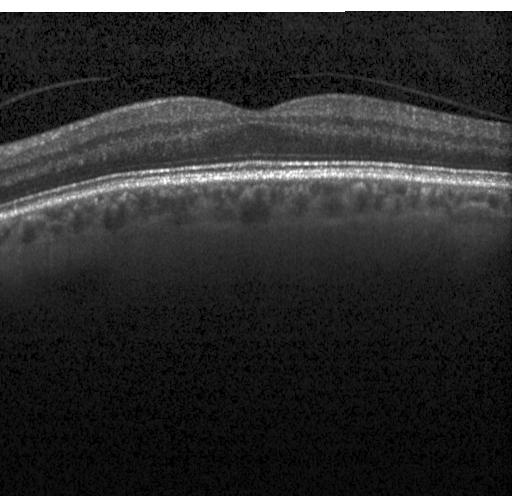

OCT line scan.
Finding: neither choroidal neovascularization, diabetic macular edema, nor drusen.